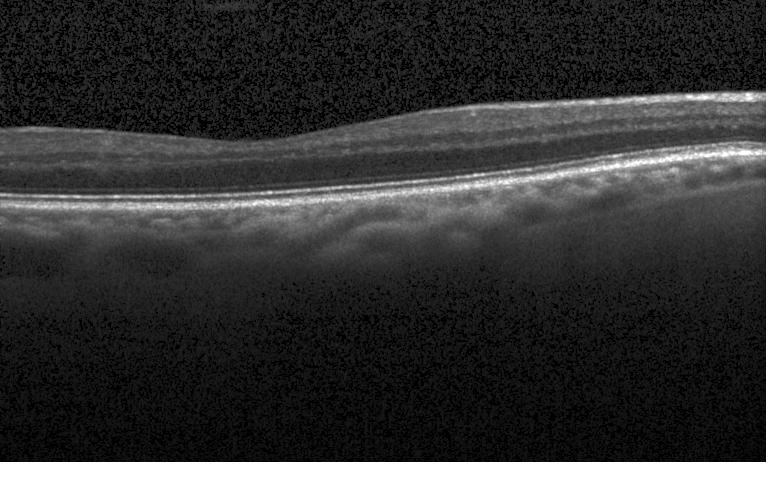

Through the macula · OCT B-scan — The scan shows no choroidal neovascularization, no diabetic macular edema, and no drusen.